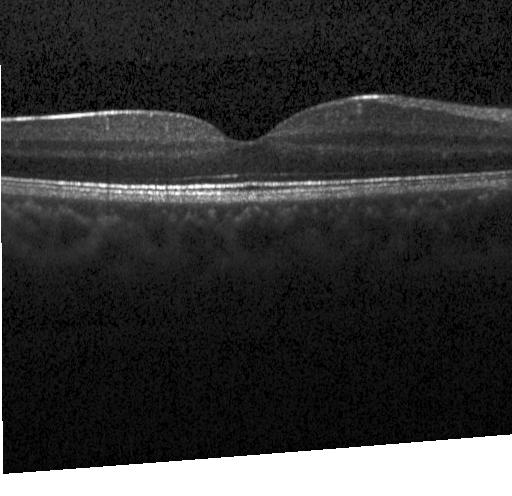

Retinal OCT cross-section
Diagnosis: no choroidal neovascularization, no diabetic macular edema, and no drusen.